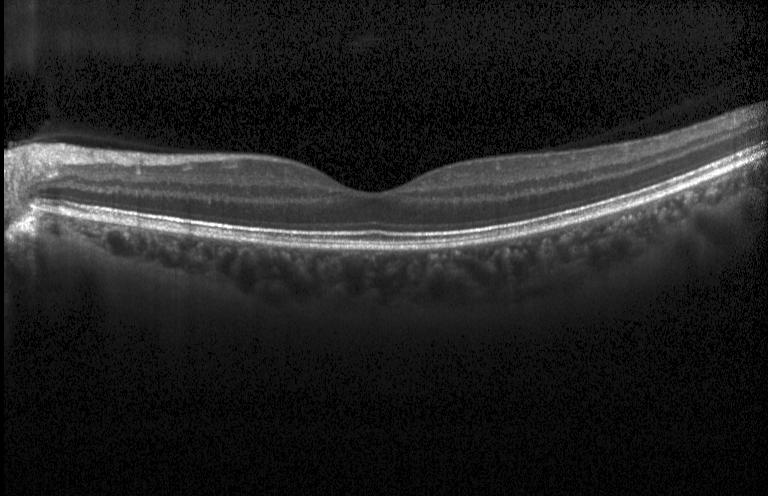 Macular scan, spectral-domain optical coherence tomography, OCT line scan, acquired on a Heidelberg Spectralis — Neither CNV, DME, nor drusen.